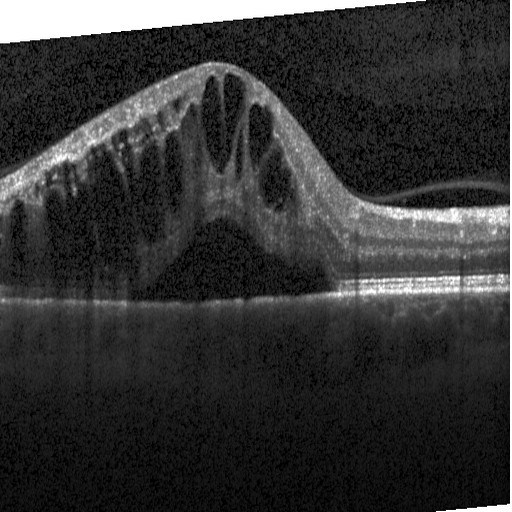
Retinal OCT B-scan.
Finding: diabetic macular edema.